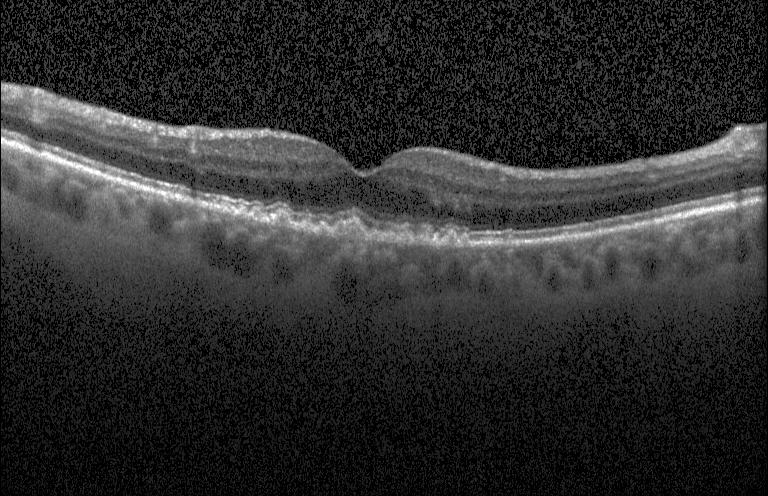 Retinal OCT B-scan — The scan shows sub-RPE drusenoid deposits.